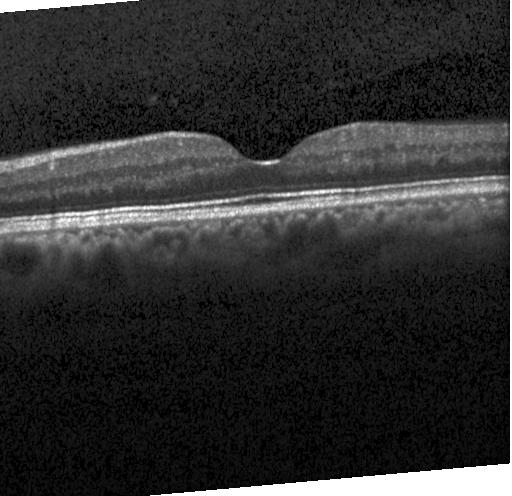 Diagnosis: no evidence of choroidal neovascularization, diabetic macular edema, or drusen.